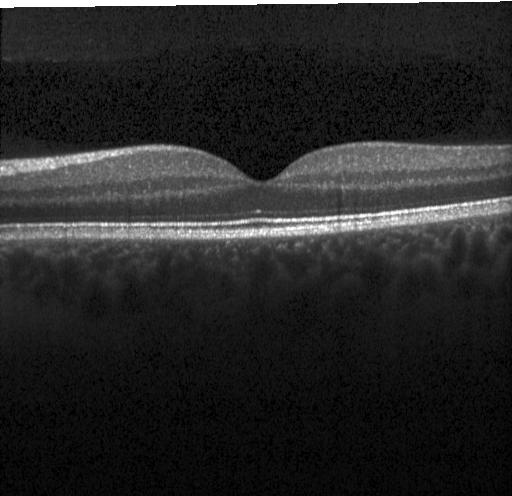

Fovea-centered. Heidelberg Spectralis. Optical coherence tomography B-scan. Spectral-domain optical coherence tomography
Neither CNV, DME, nor drusen.